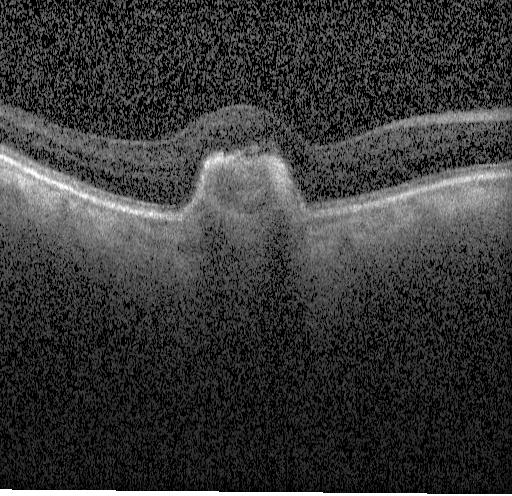
Optical coherence tomography B-scan. Macular scan. Heidelberg Spectralis OCT system.
Choroidal neovascularization.